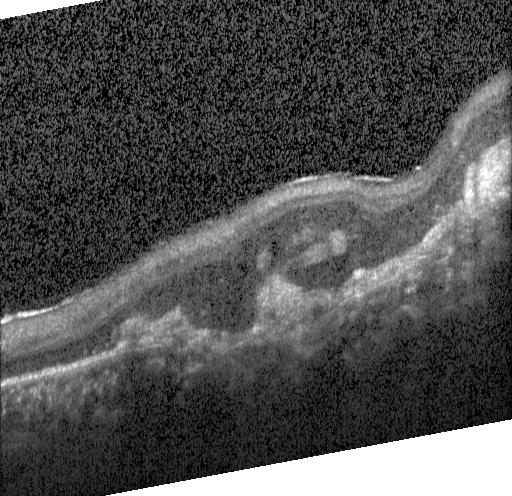
Optical coherence tomography scan; Heidelberg Spectralis; SD-OCT
Macular OCT: a choroidal neovascular membrane.